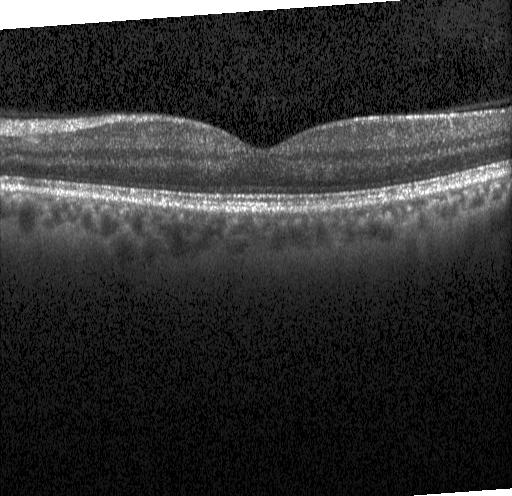

Centered on the fovea; retinal OCT B-scan; spectral-domain optical coherence tomography — Impression: neither CNV, DME, nor drusen.